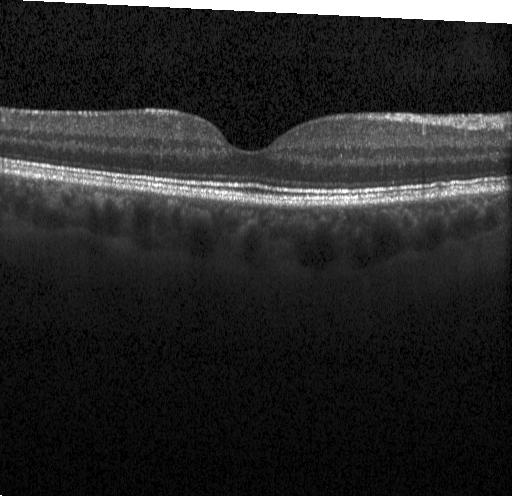 The scan shows no choroidal neovascularization, no diabetic macular edema, and no drusen.